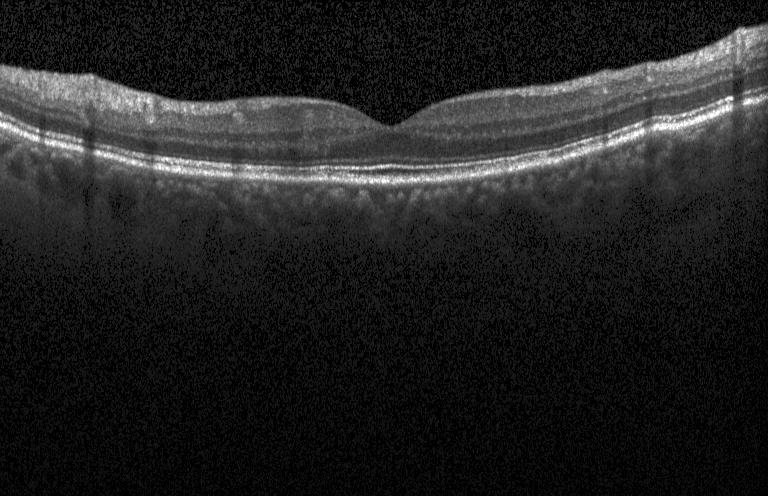
OCT B-scan · instrument: Heidelberg Spectralis · spectral-domain optical coherence tomography — Diagnosis: neither choroidal neovascularization, diabetic macular edema, nor drusen.